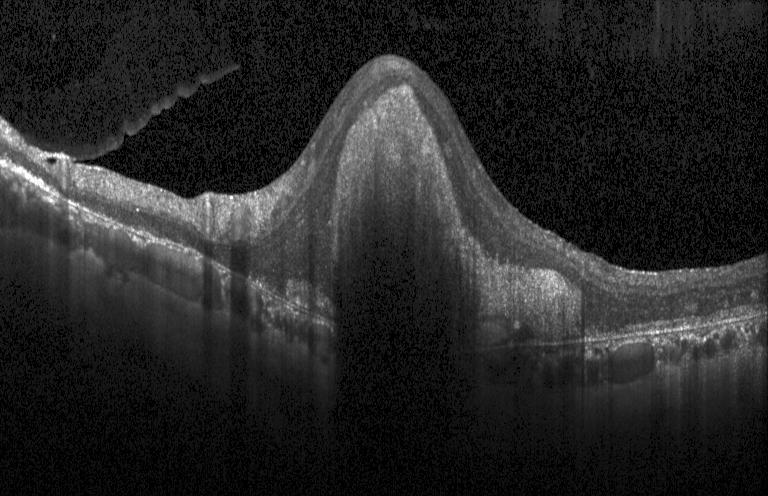 Dx: CNV.